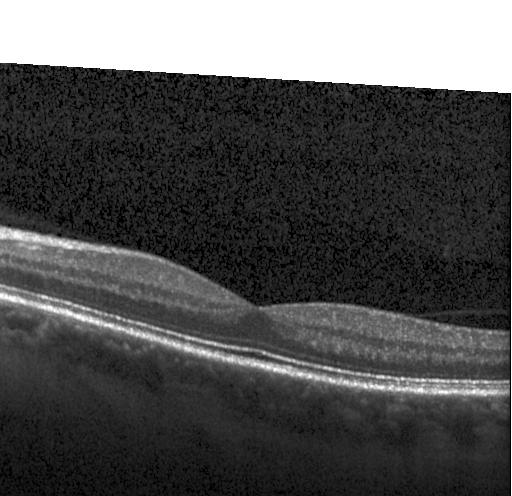 SD-OCT; fovea-centered; retinal OCT B-scan. Dx: no CNV, DME, or drusen.